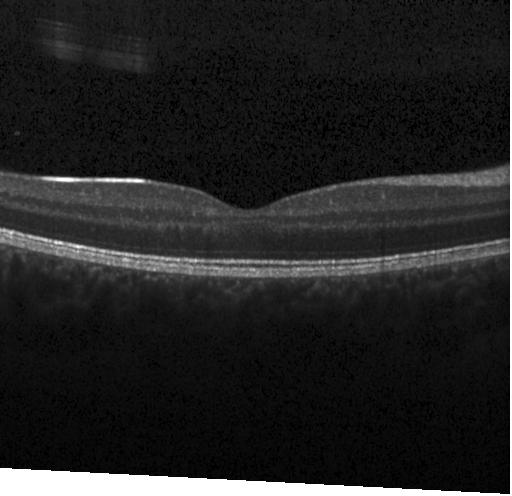
Dx: no choroidal neovascularization, no diabetic macular edema, and no drusen.